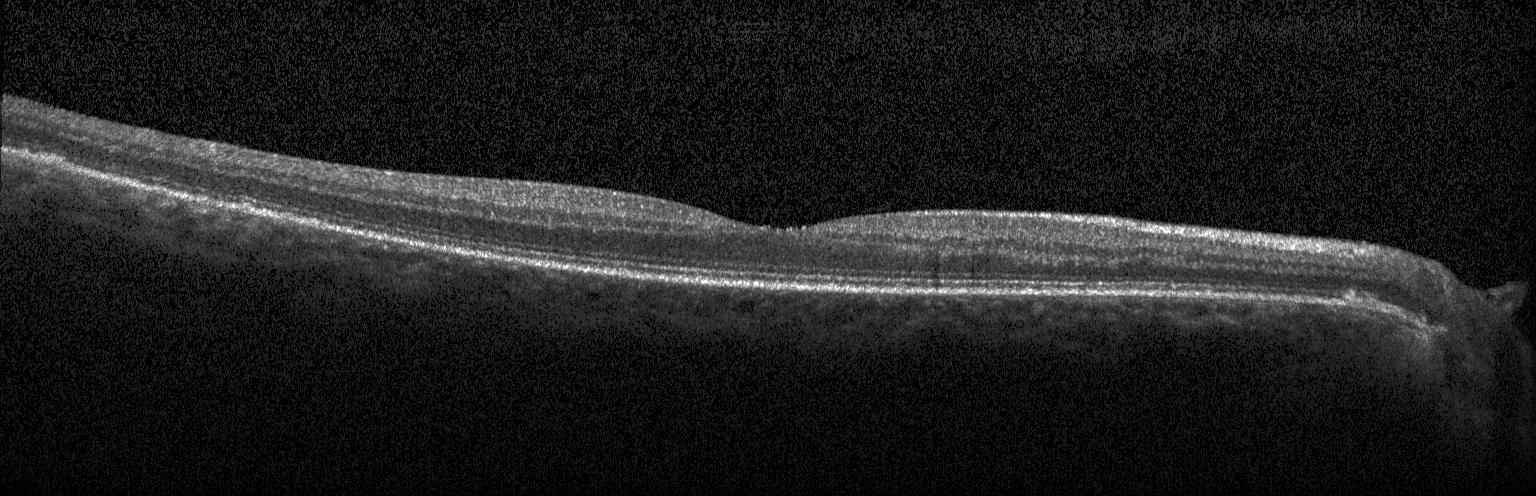 Impression: no evidence of CNV, DME, or drusen.